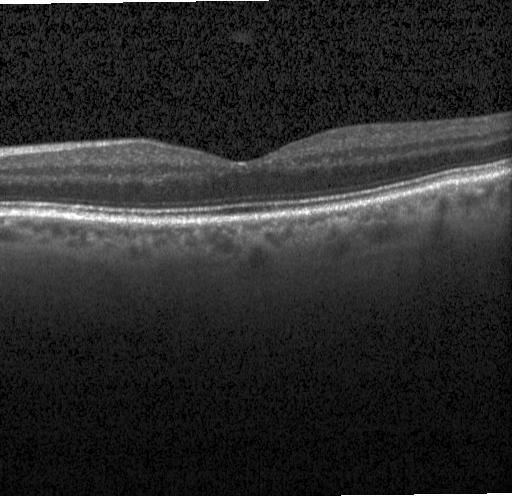

Assessment: no CNV, DME, or drusen.